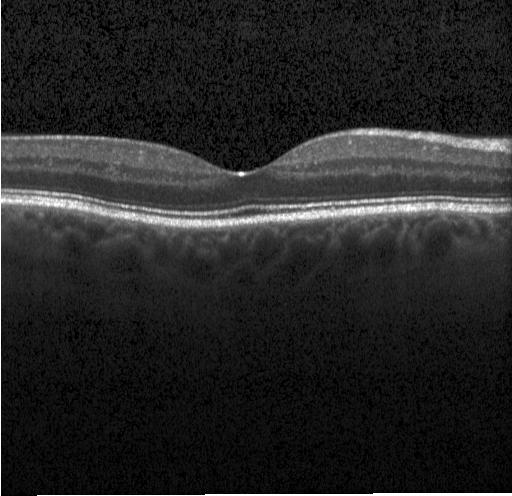

OCT line scan, spectral-domain optical coherence tomography, fovea-centered, instrument: Heidelberg Spectralis.
Dx: no evidence of choroidal neovascularization, diabetic macular edema, or drusen.